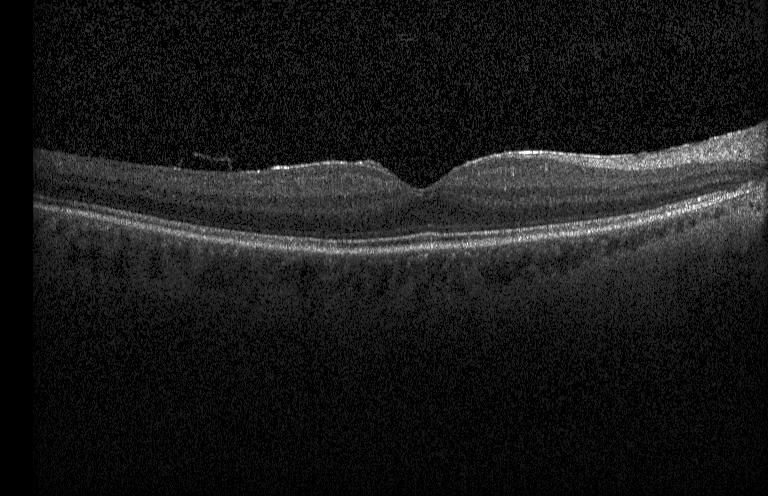 Retinal OCT cross-section. Diagnosis: no choroidal neovascularization, diabetic macular edema, or drusen.